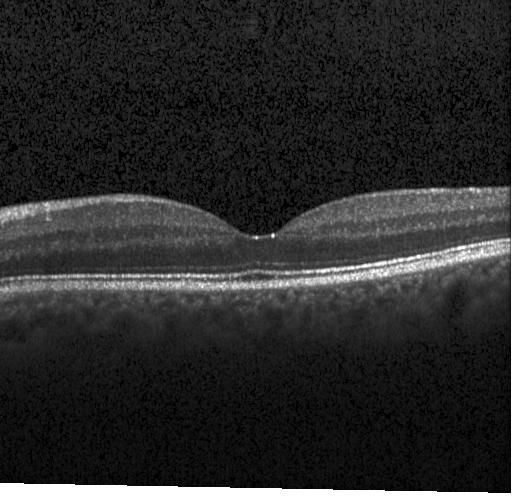

OCT B-scan showing no evidence of choroidal neovascularization, diabetic macular edema, or drusen.